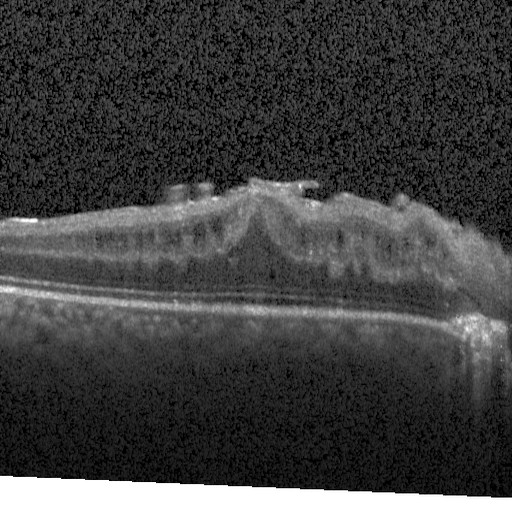 OCT line scan.
Impression: diabetic macular edema.